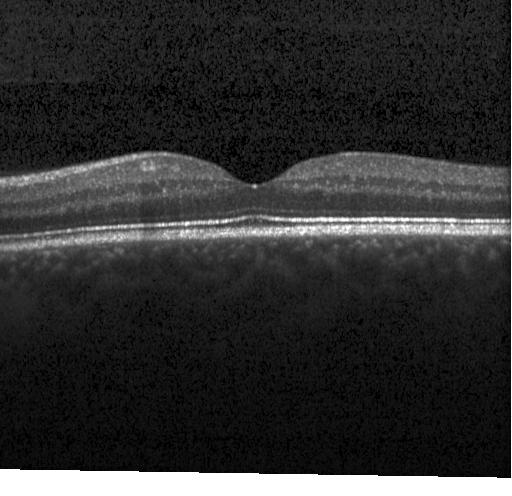 Spectral-domain OCT · OCT line scan · Heidelberg Spectralis OCT system. OCT finding: no evidence of CNV, DME, or drusen.